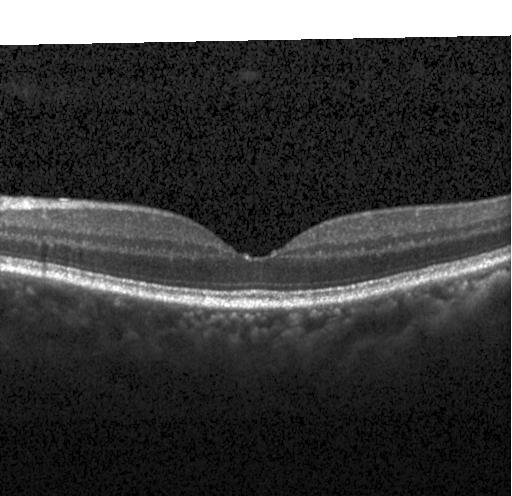

This B-scan demonstrates neither choroidal neovascularization, diabetic macular edema, nor drusen.